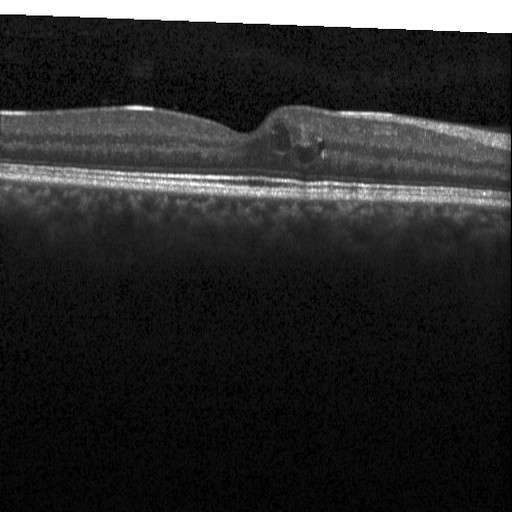 Optical coherence tomography scan
Finding: DME.